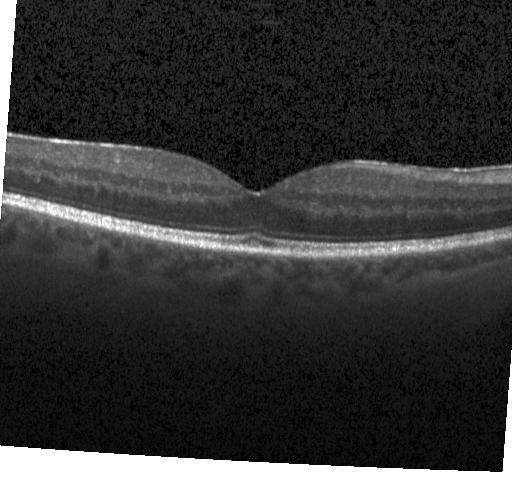

Fovea-centered · OCT B-scan · Heidelberg Spectralis OCT system
No choroidal neovascularization, diabetic macular edema, or drusen.